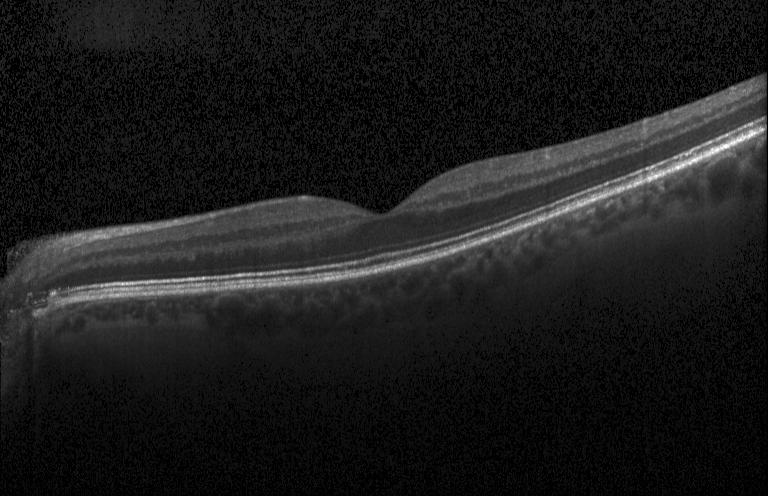
Retinal OCT cross-section; Heidelberg Spectralis; spectral-domain optical coherence tomography.
Finding: no choroidal neovascularization, no diabetic macular edema, and no drusen.